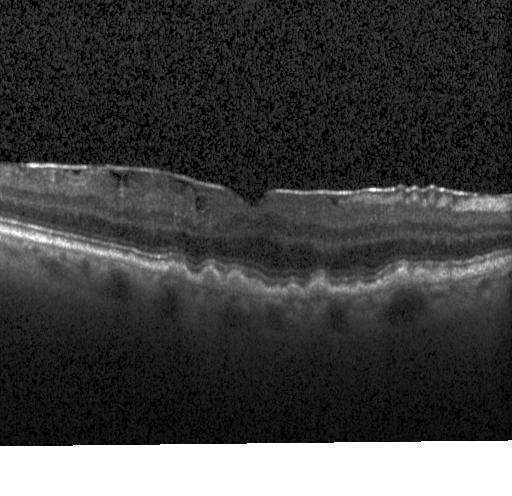
This B-scan demonstrates multiple drusen.